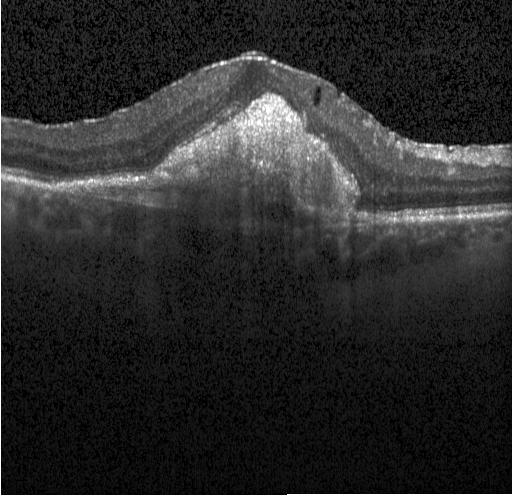

Optical coherence tomography scan. Diagnosis: a choroidal neovascular membrane.